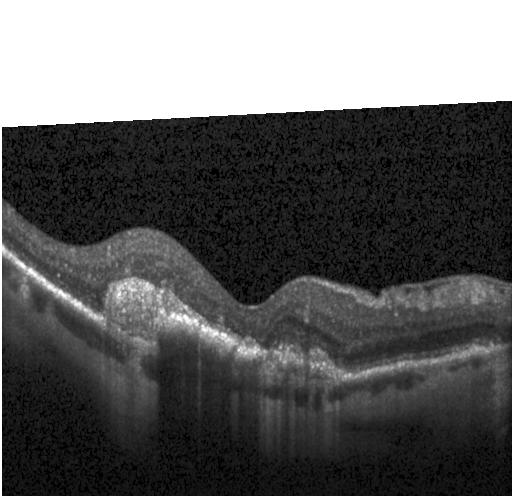 Macular OCT demonstrating a choroidal neovascular membrane.